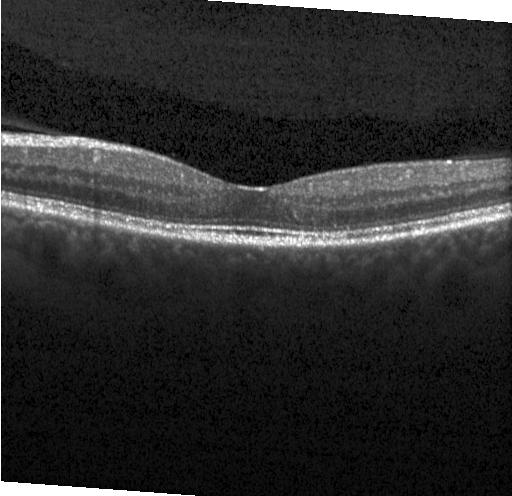 OCT B-scan showing neither choroidal neovascularization, diabetic macular edema, nor drusen.